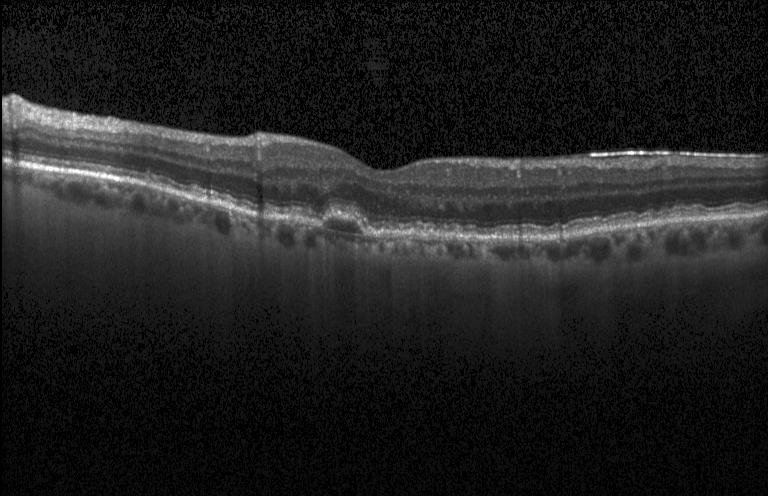

Finding: a choroidal neovascular membrane.